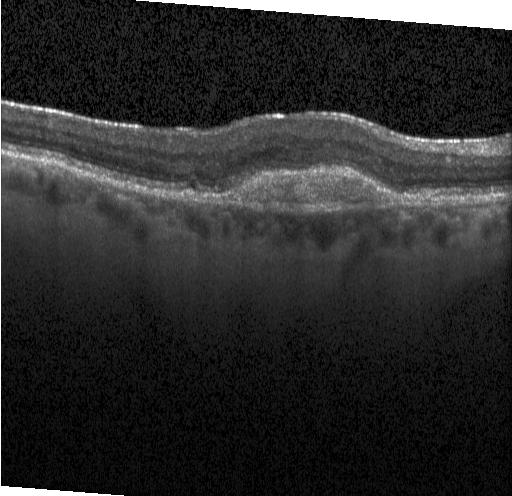
Dx: choroidal neovascularization.